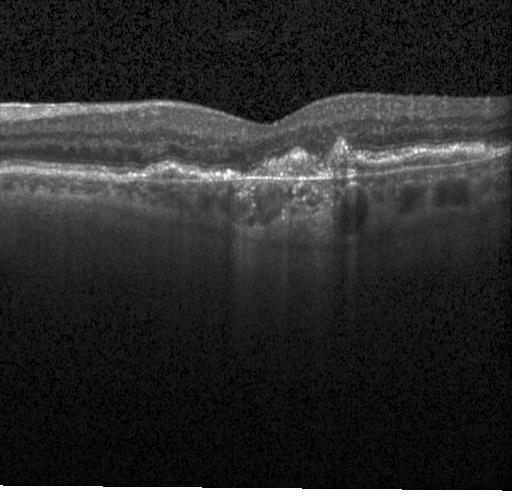
Diagnosis: CNV.